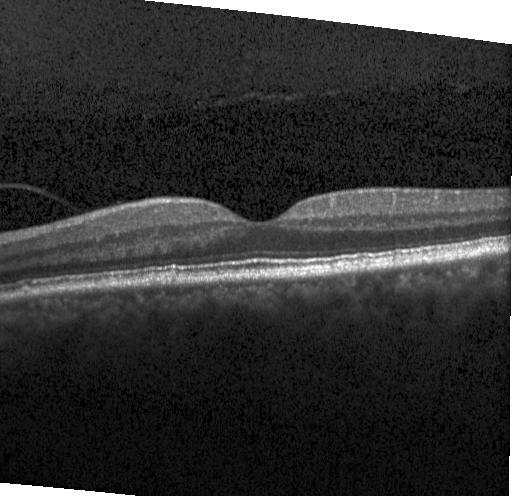
Centered on the fovea · retinal OCT cross-section · spectral-domain optical coherence tomography · Heidelberg Spectralis OCT system.
Macular OCT: no choroidal neovascularization, diabetic macular edema, or drusen.